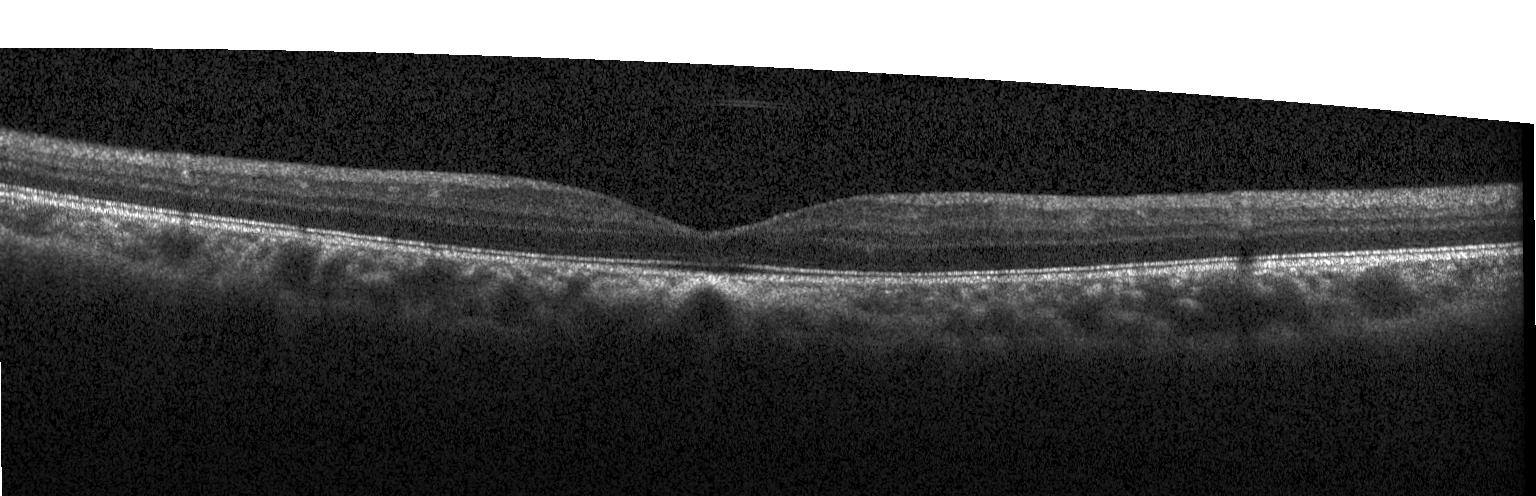 Dx: no choroidal neovascularization, no diabetic macular edema, and no drusen.